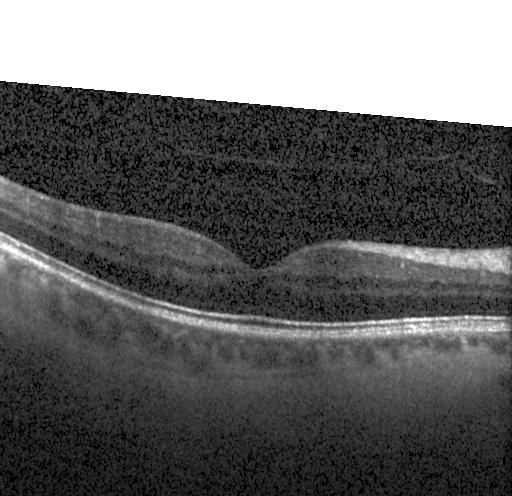

Retinal OCT B-scan · macular scan. Dx: neither CNV, DME, nor drusen.